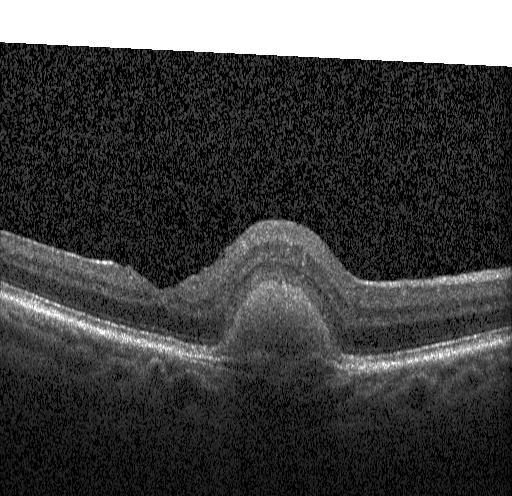 Retinal OCT B-scan.
OCT finding: a choroidal neovascular membrane.